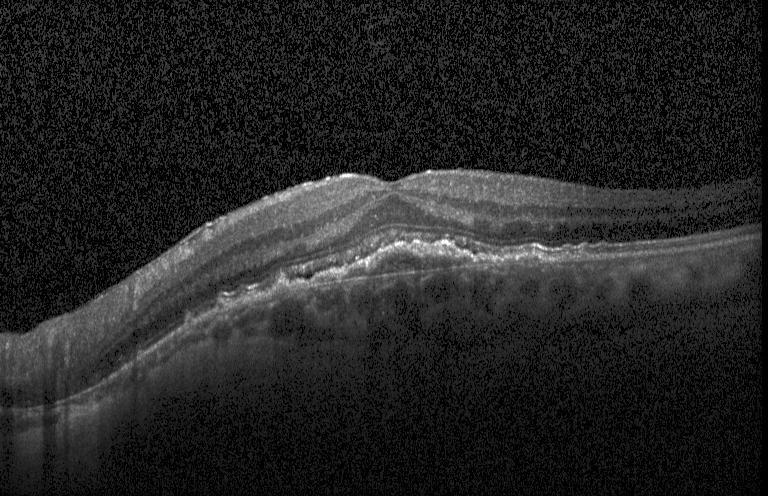

Spectral-domain optical coherence tomography · retinal OCT cross-section · instrument: Heidelberg Spectralis — Dx: CNV.